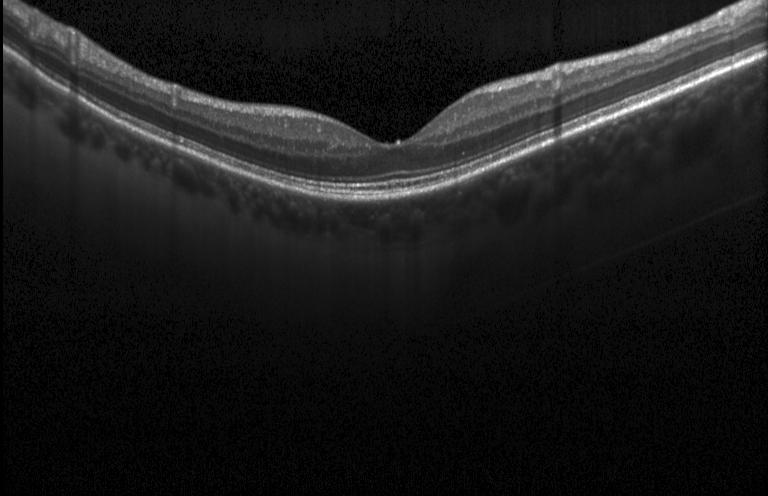 Dx: no choroidal neovascularization, no diabetic macular edema, and no drusen.